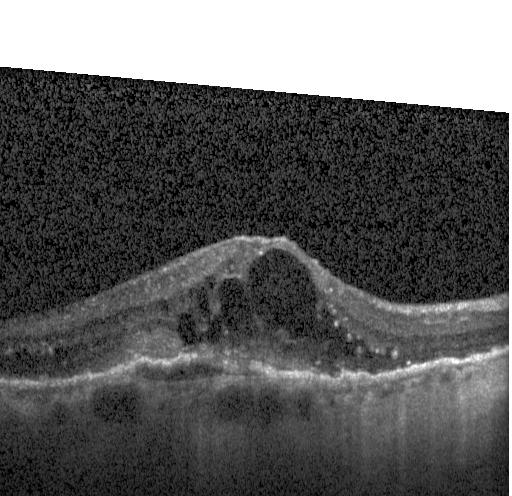
Choroidal neovascularization (CNV).